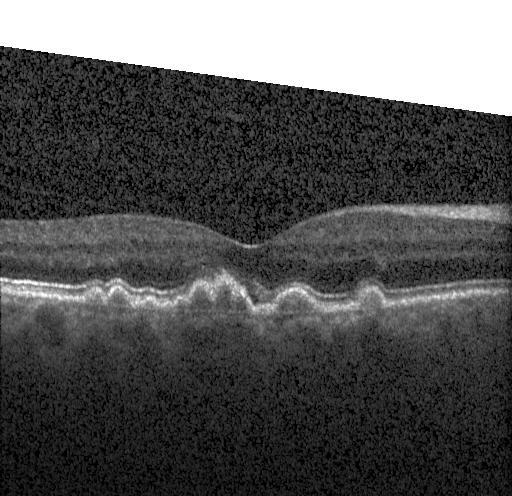

This B-scan demonstrates sub-RPE drusenoid deposits.